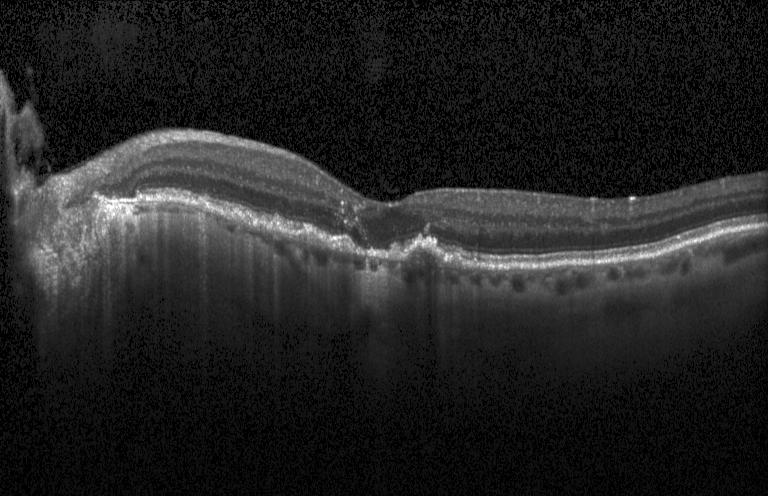 OCT finding: multiple drusen.